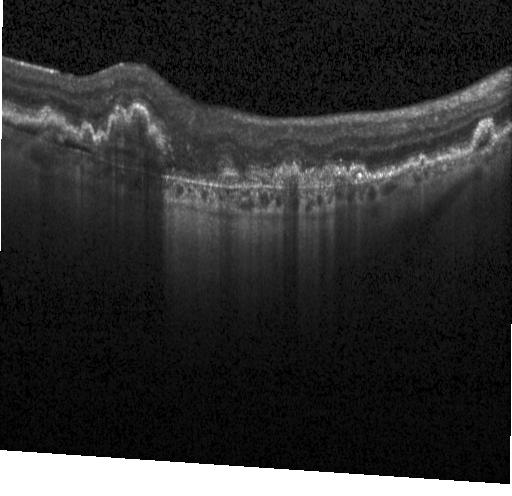

Instrument: Heidelberg Spectralis. Retinal OCT B-scan. Fovea-centered. SD-OCT — Impression: a choroidal neovascular membrane.